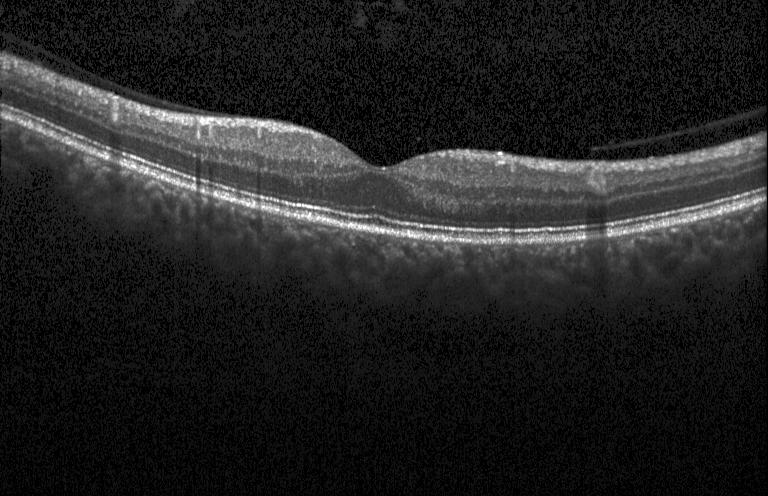 Retinal OCT cross-section. This B-scan demonstrates no evidence of CNV, DME, or drusen.